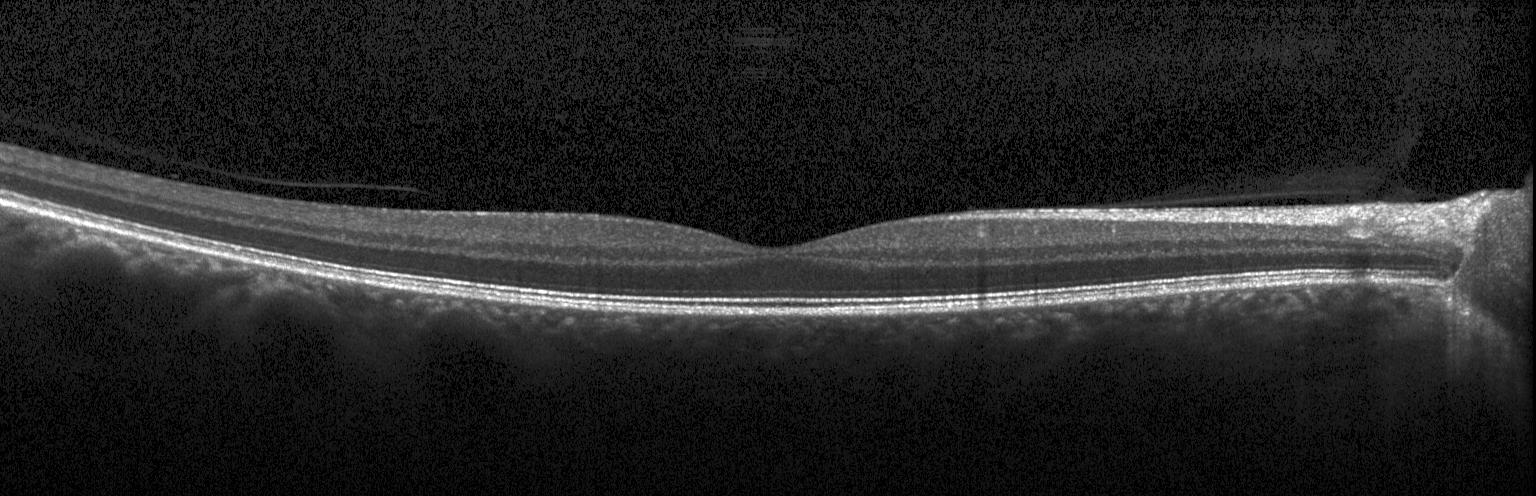
No evidence of choroidal neovascularization, diabetic macular edema, or drusen.